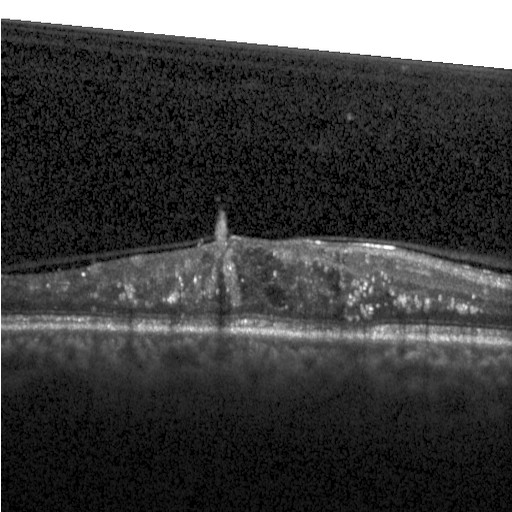
Impression: DME.